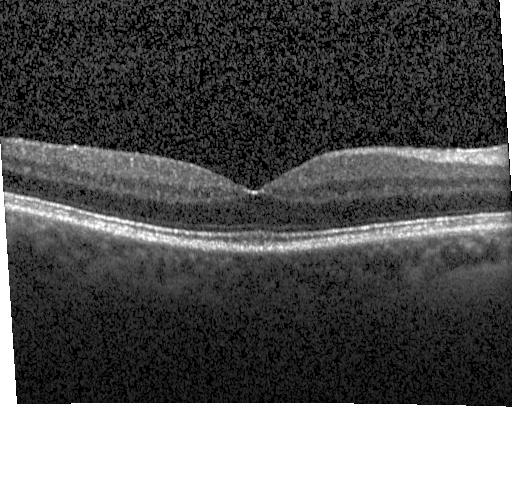
Spectral-domain OCT; fovea-centered; optical coherence tomography scan; acquired on a Heidelberg Spectralis.
The scan shows no CNV, no DME, and no drusen.